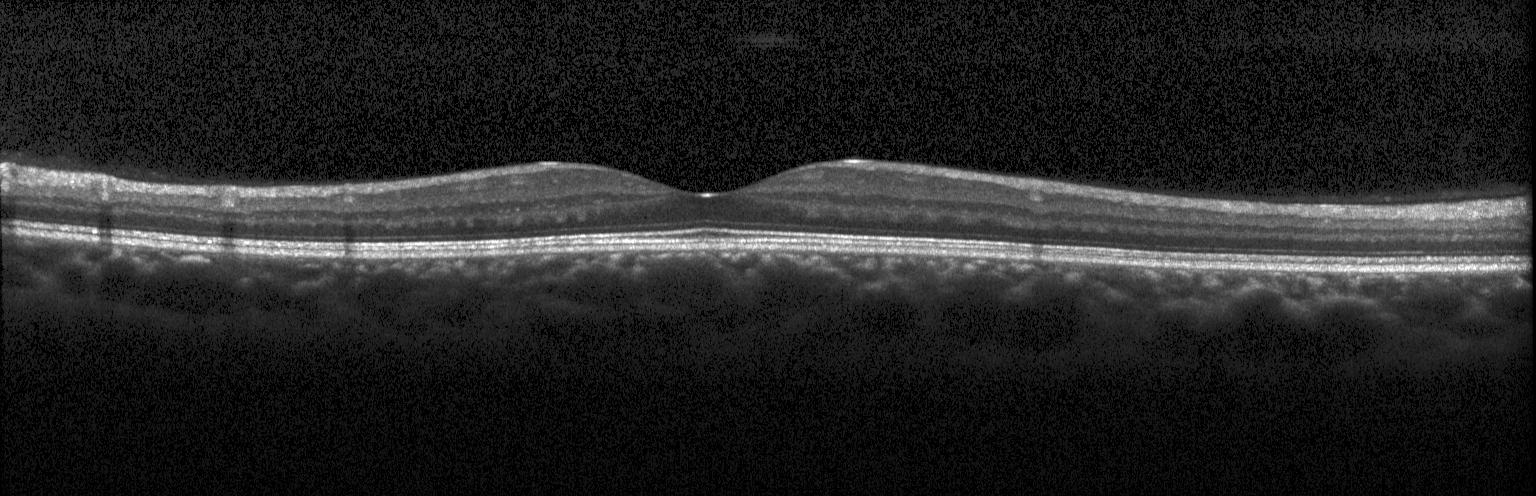

Heidelberg Spectralis, OCT line scan, spectral-domain optical coherence tomography — Impression: no evidence of choroidal neovascularization, diabetic macular edema, or drusen.